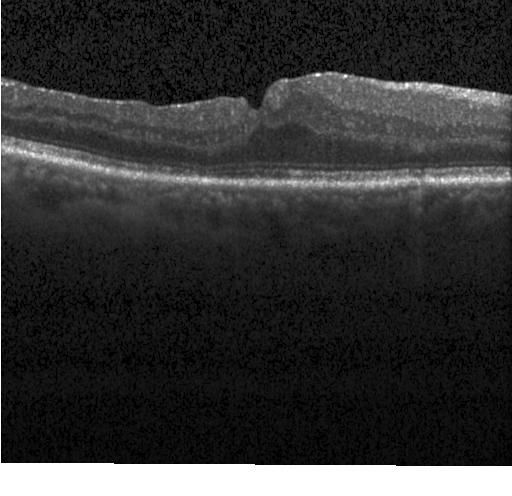 Diagnosis: no choroidal neovascularization, diabetic macular edema, or drusen.